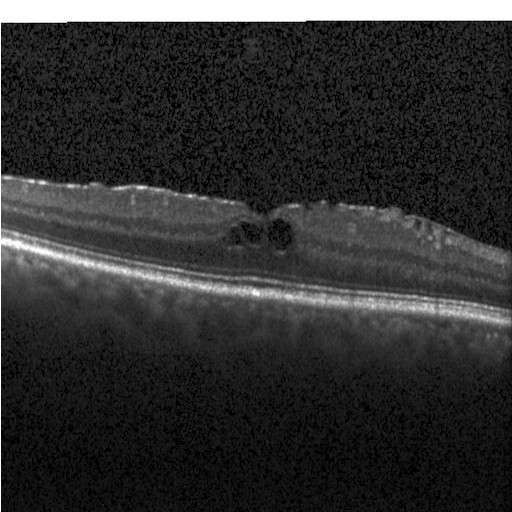
Assessment: DME.